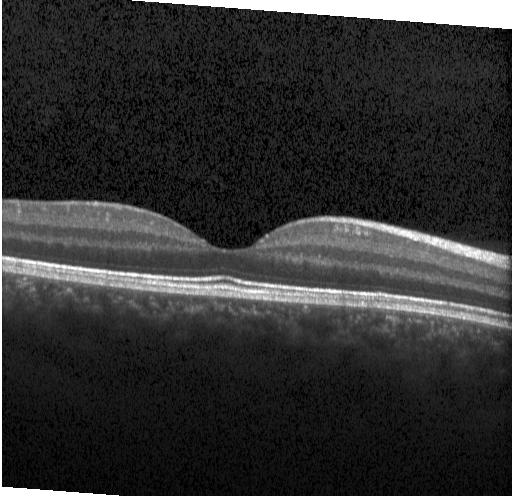

Retinal OCT B-scan — No choroidal neovascularization, no diabetic macular edema, and no drusen.